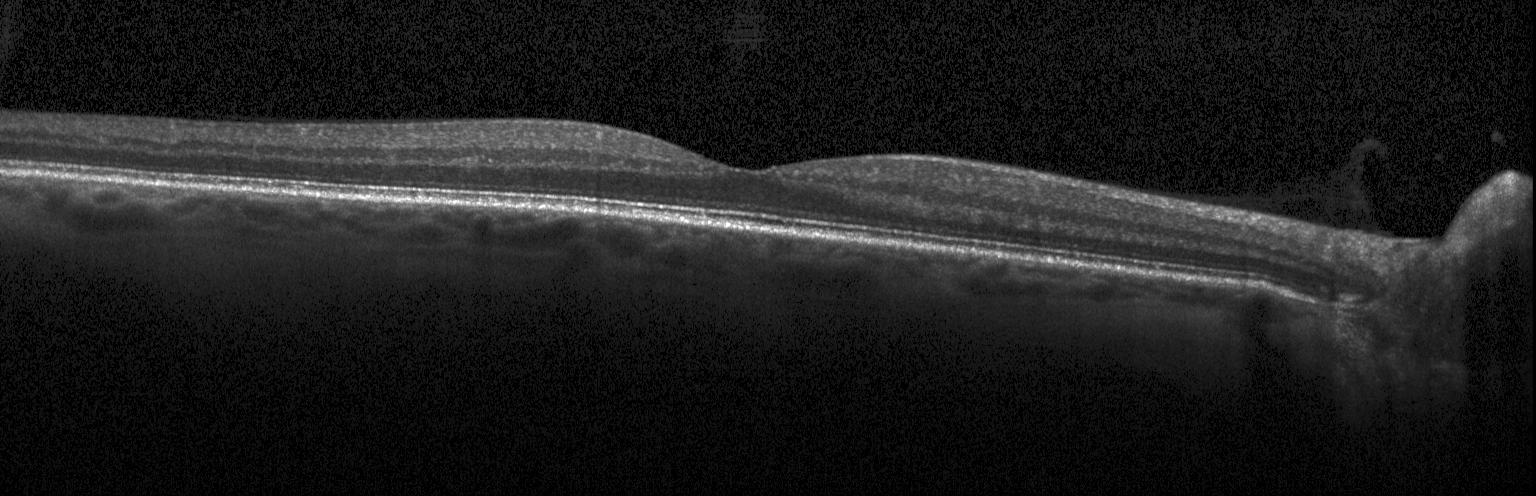 Retinal OCT cross-section · spectral-domain optical coherence tomography.
Finding: no CNV, no DME, and no drusen.